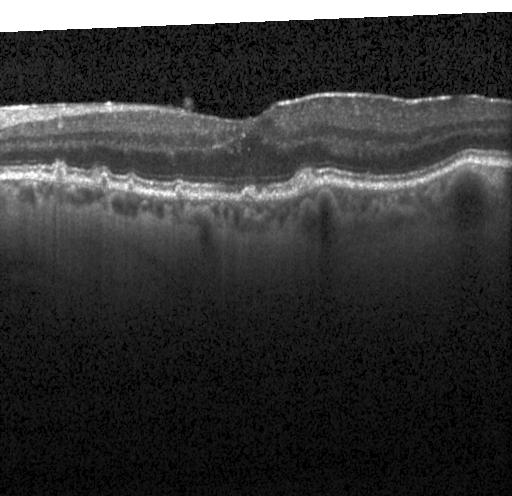 Impression: multiple drusen.